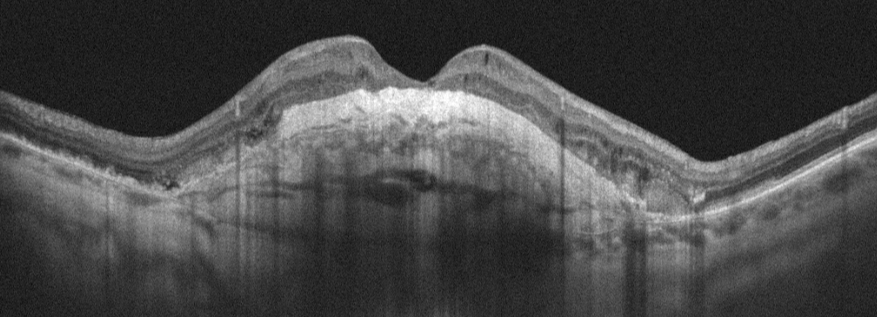

Macular scan · acquired on an Optovue Avanti RTVue XR · retinal OCT cross-section. Diagnosis: AMD.